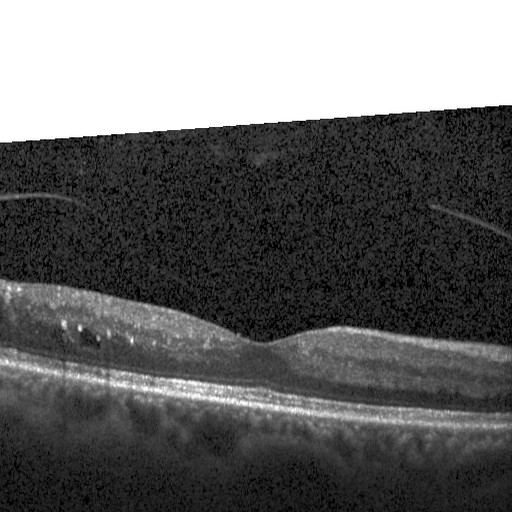 Impression: DME.